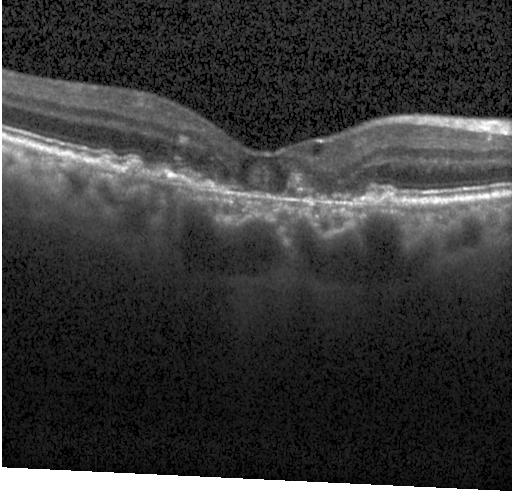

OCT B-scan, centered on the fovea. Impression: choroidal neovascularization (CNV).